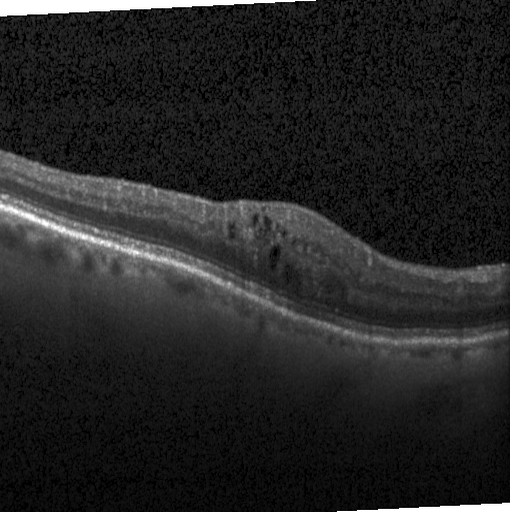
Spectral-domain optical coherence tomography, OCT B-scan, macular scan.
Impression: DME.